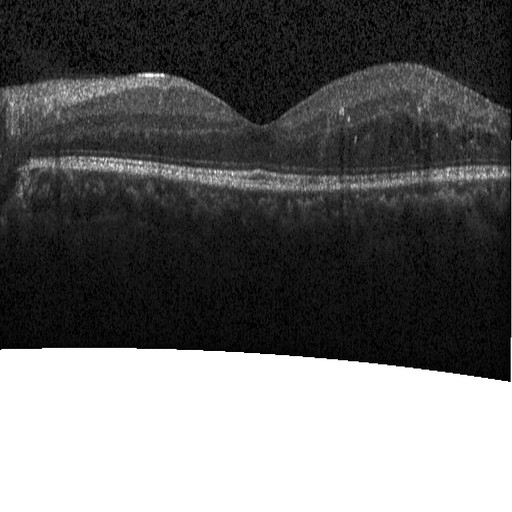

Spectral-domain optical coherence tomography. Optical coherence tomography scan. Instrument: Heidelberg Spectralis.
This B-scan demonstrates diabetic macular edema.